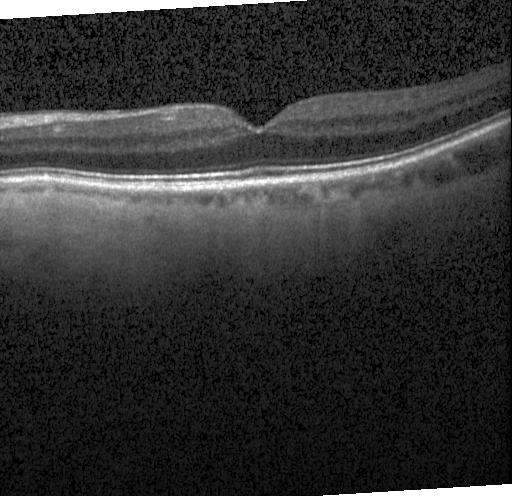 Assessment: no evidence of CNV, DME, or drusen.